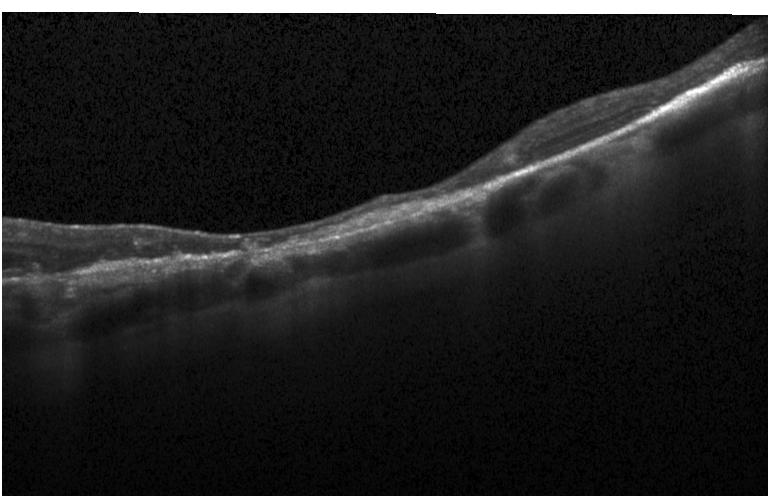
Macular OCT: a choroidal neovascular membrane.